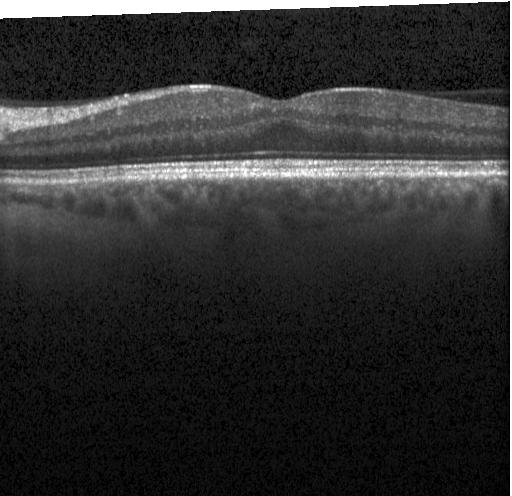

Acquired on a Heidelberg Spectralis · spectral-domain optical coherence tomography · optical coherence tomography scan — Finding: no choroidal neovascularization, no diabetic macular edema, and no drusen.